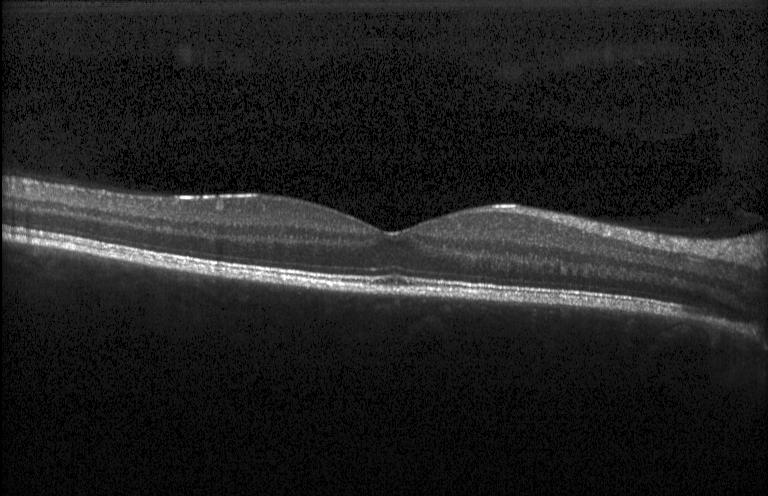

OCT line scan. Centered on the fovea. Spectral-domain OCT
Macular OCT: no CNV, DME, or drusen.